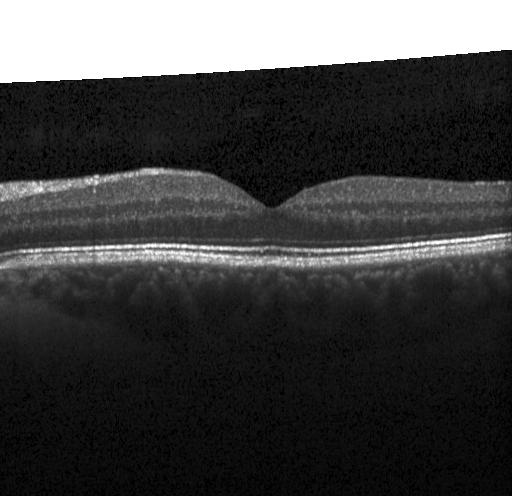 OCT B-scan, spectral-domain optical coherence tomography, horizontal scan through the fovea.
Finding: no evidence of choroidal neovascularization, diabetic macular edema, or drusen.